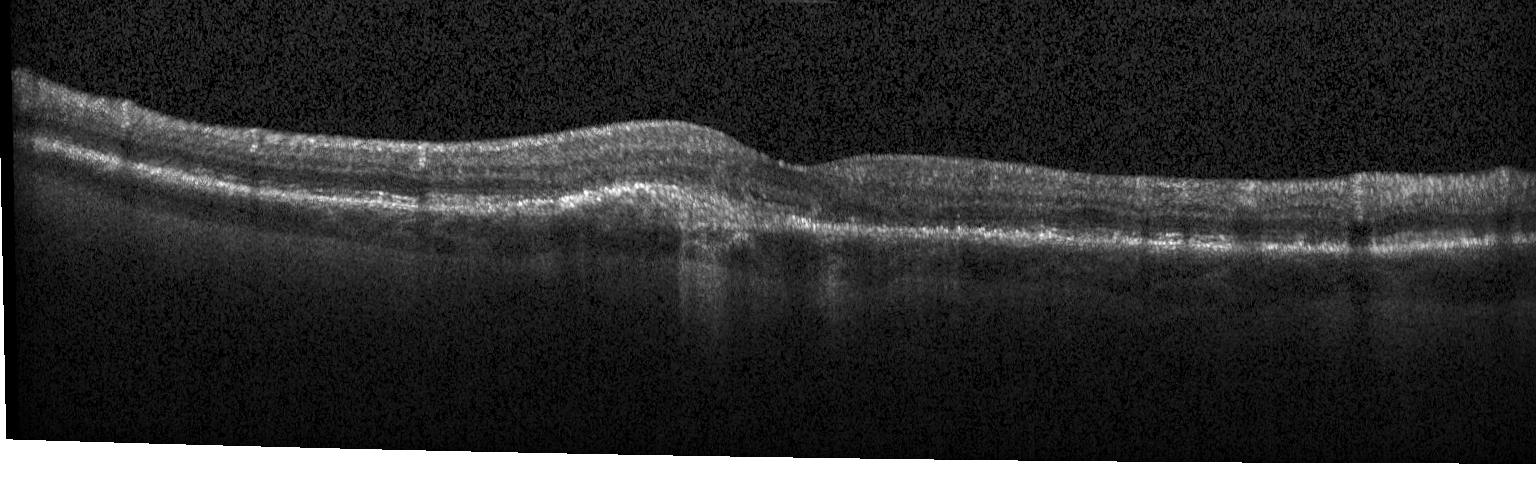 Impression: a choroidal neovascular membrane.